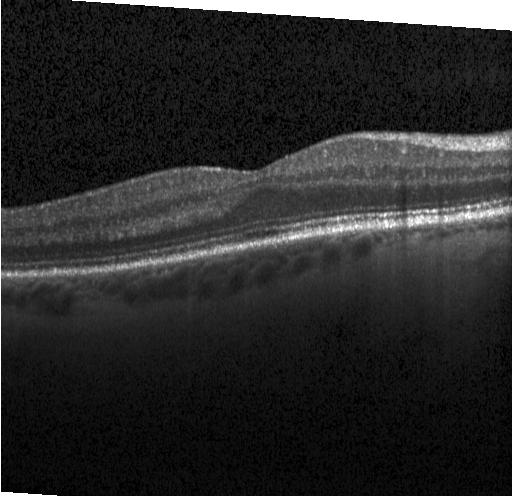

Optical coherence tomography scan — OCT finding: no CNV, DME, or drusen.